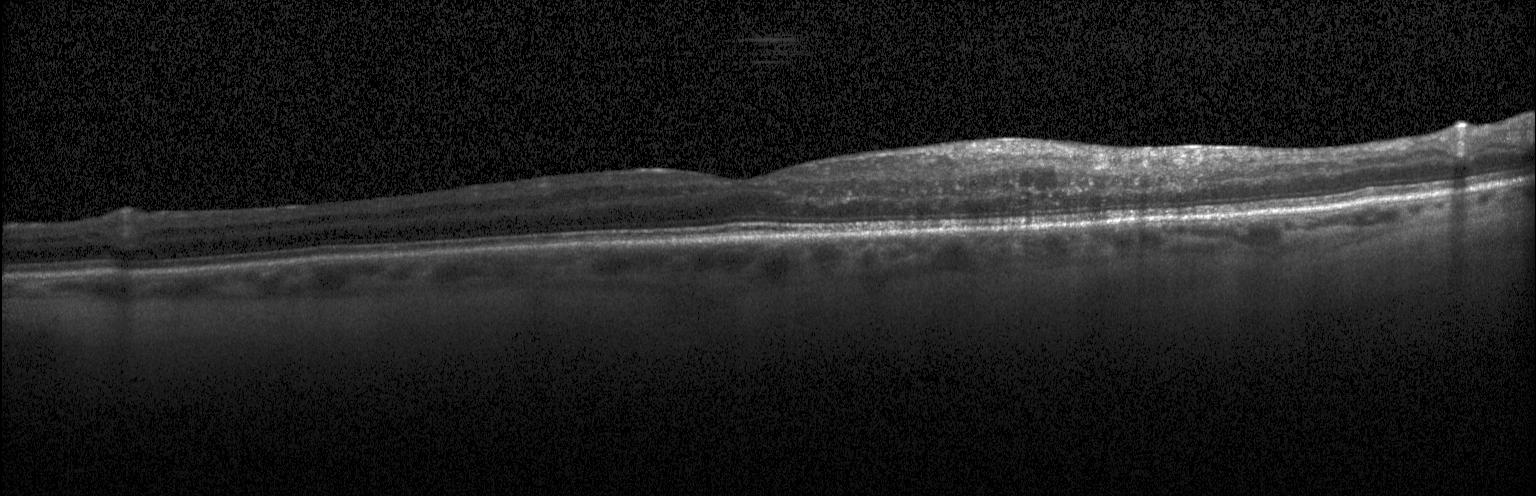
Acquired on a Heidelberg Spectralis · retinal OCT cross-section — This B-scan demonstrates diabetic macular edema.